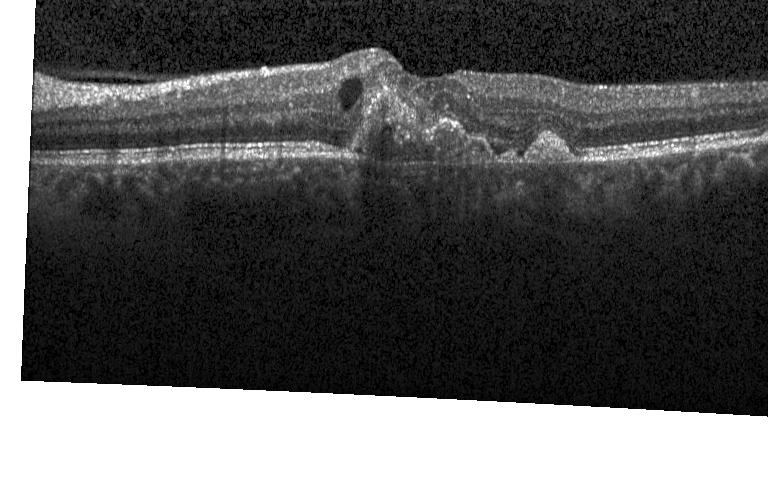

Heidelberg Spectralis OCT system; OCT line scan; spectral-domain optical coherence tomography — A choroidal neovascular membrane.